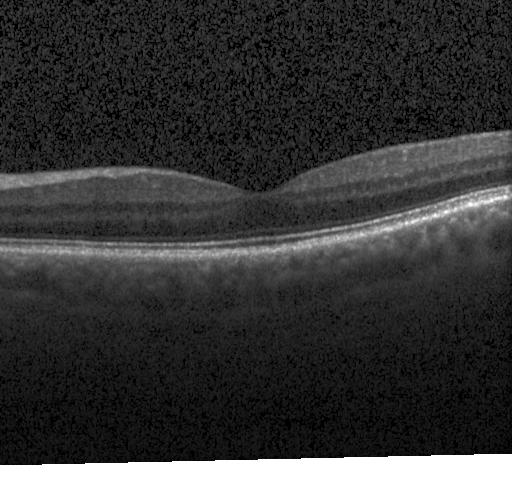 Fovea-centered. Retinal OCT B-scan
This B-scan demonstrates no CNV, DME, or drusen.